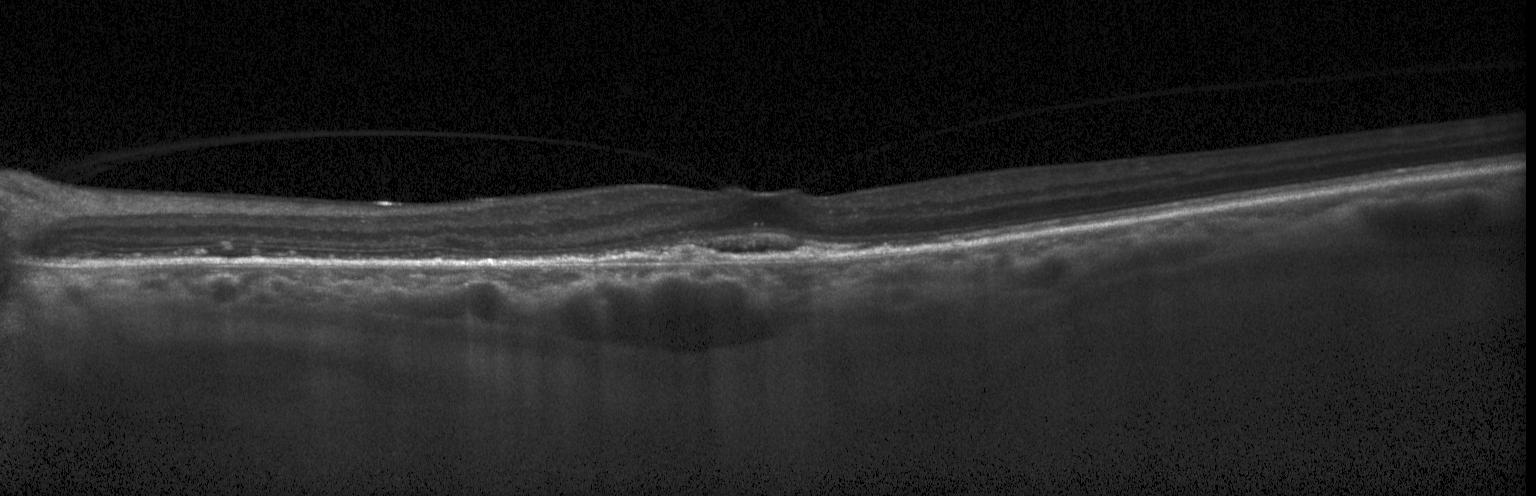

Spectral-domain optical coherence tomography; fovea-centered; optical coherence tomography B-scan
Impression: a choroidal neovascular membrane.